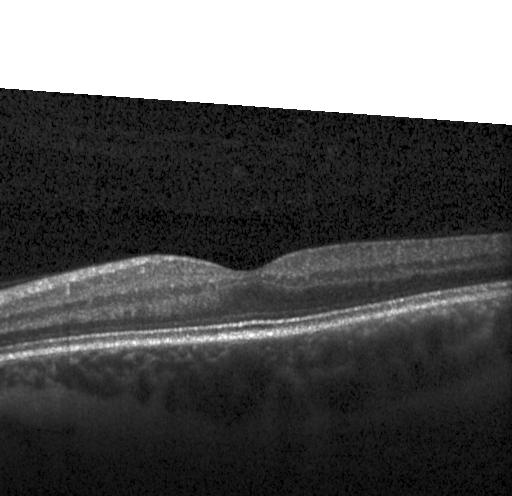 Heidelberg Spectralis OCT system; SD-OCT; centered on the fovea; OCT B-scan.
Finding: no CNV, no DME, and no drusen.